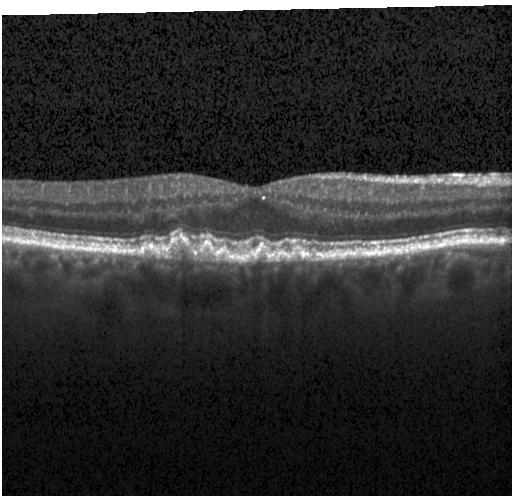

Macular OCT: sub-RPE drusenoid deposits.